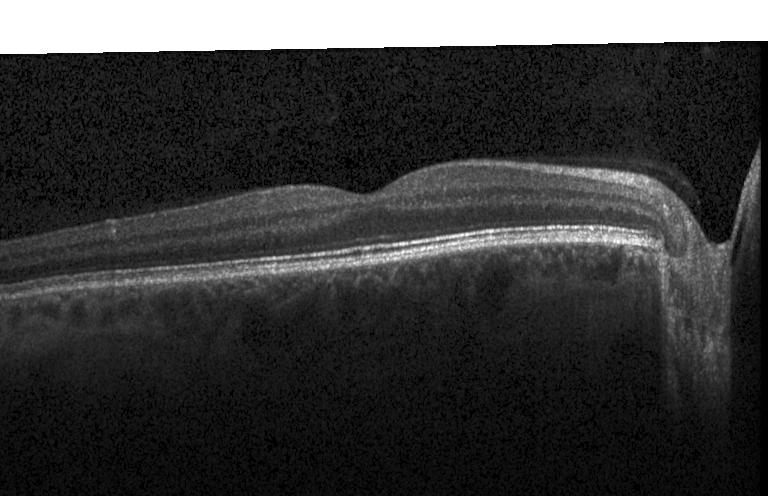

The scan shows no choroidal neovascularization, diabetic macular edema, or drusen.